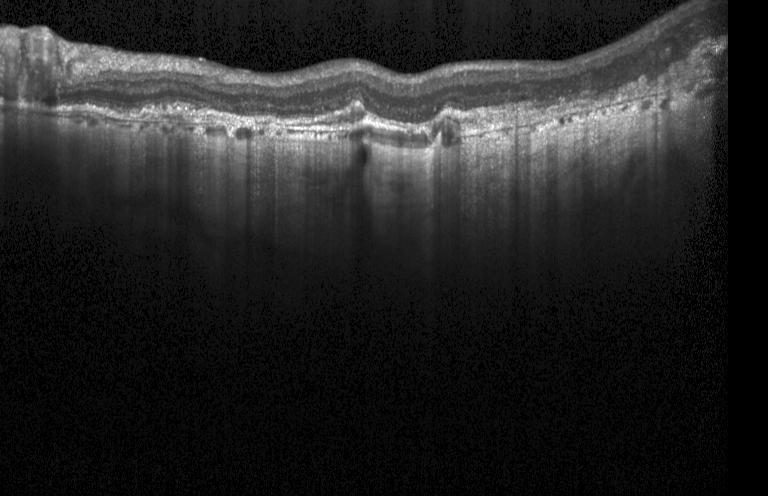
Heidelberg Spectralis, retinal OCT B-scan — OCT finding: choroidal neovascularization (CNV).